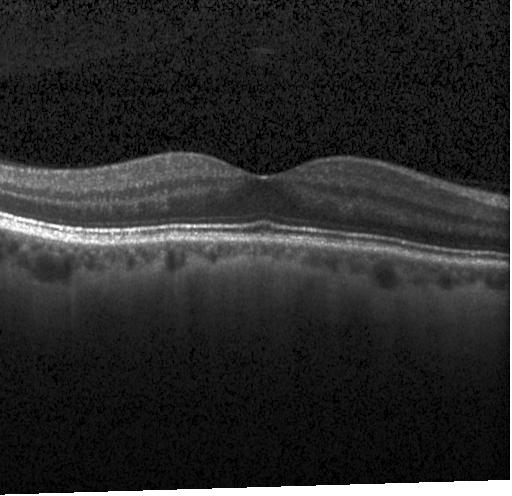 OCT B-scan showing no CNV, no DME, and no drusen.